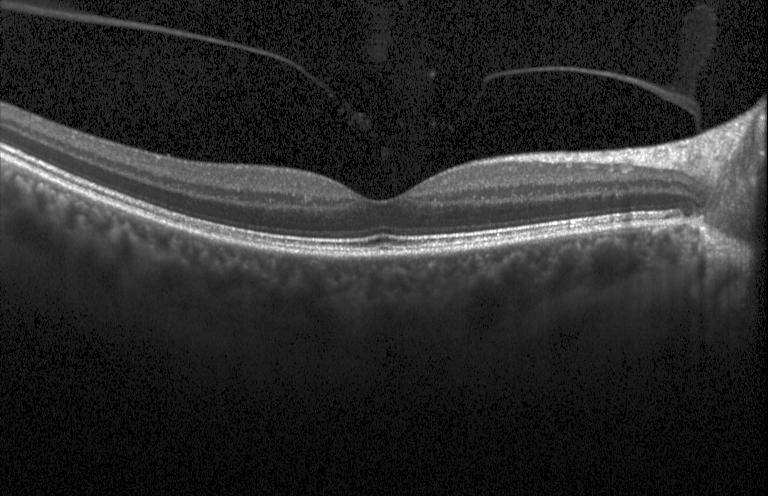
Macular scan. Optical coherence tomography B-scan. Spectral-domain optical coherence tomography. Instrument: Heidelberg Spectralis — Diagnosis: no evidence of CNV, DME, or drusen.